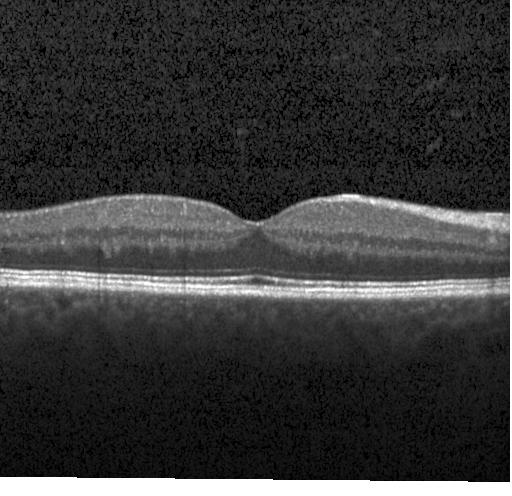 Acquired on a Heidelberg Spectralis. Retinal OCT B-scan. Diagnosis: no evidence of choroidal neovascularization, diabetic macular edema, or drusen.